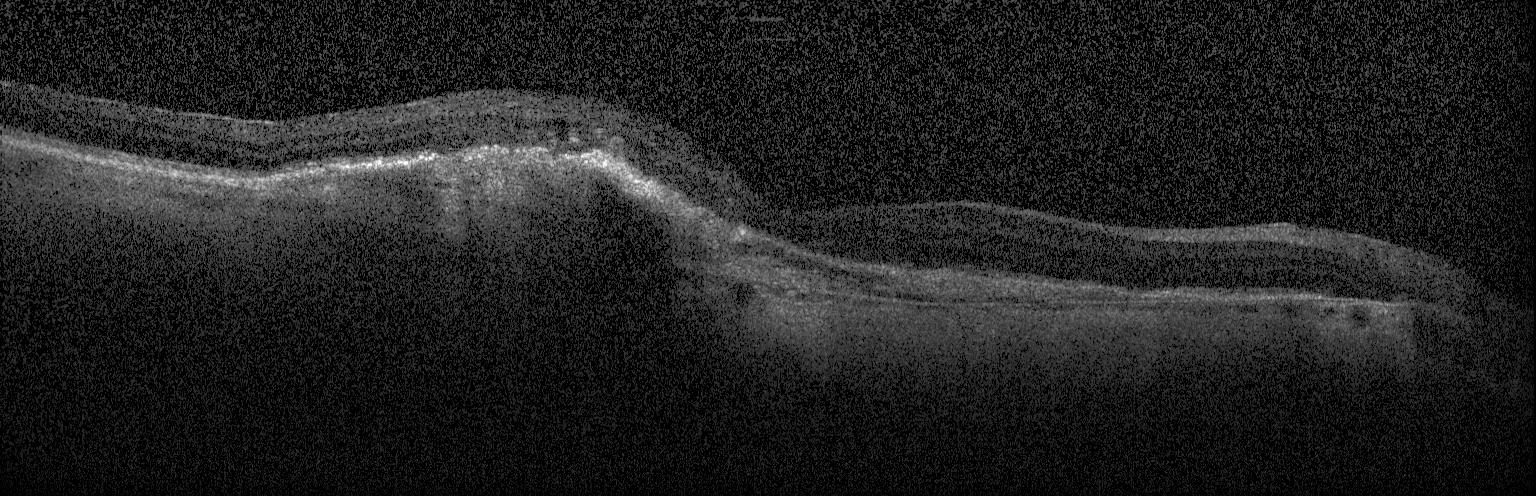 Finding: a choroidal neovascular membrane.